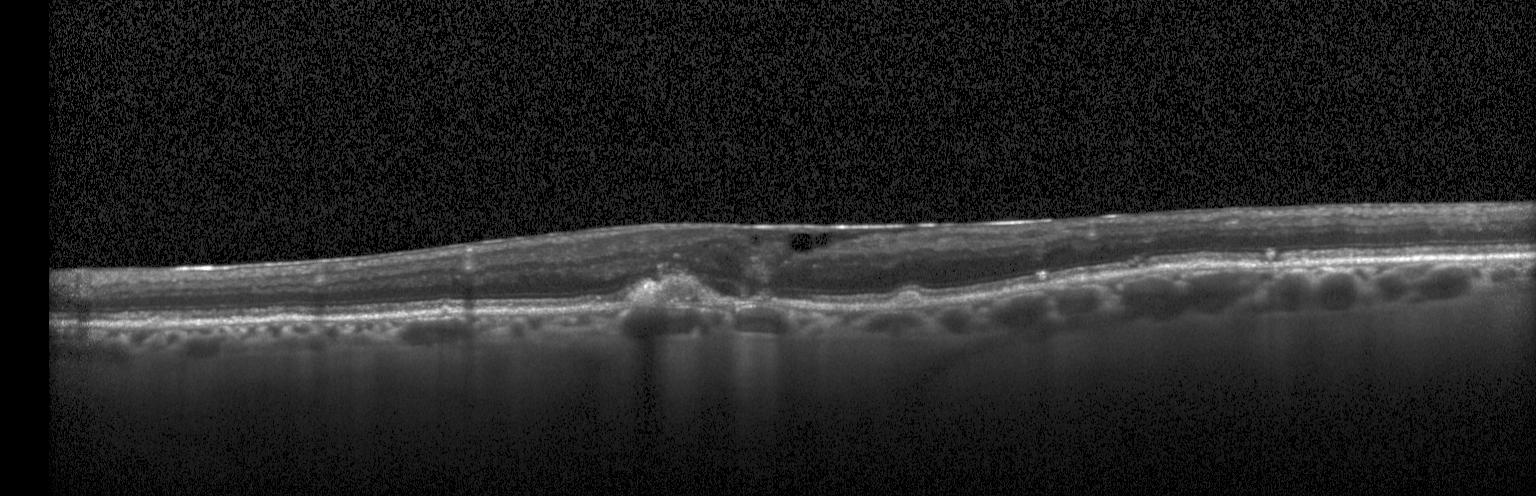 Dx: choroidal neovascularization (CNV).